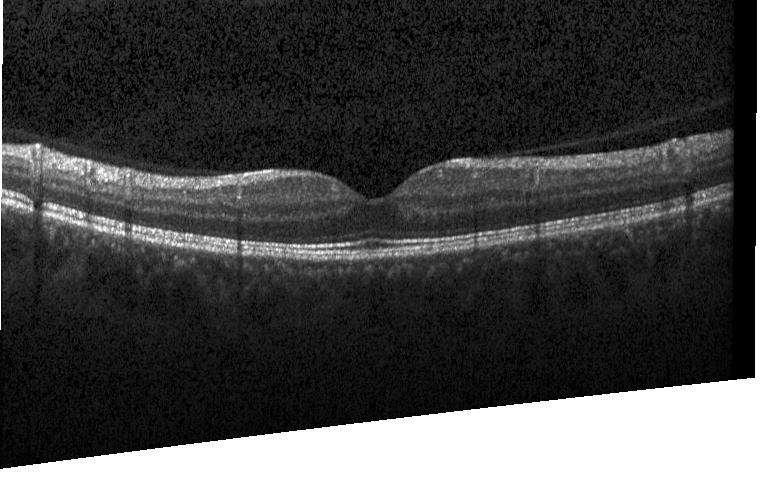

Impression: no CNV, no DME, and no drusen.